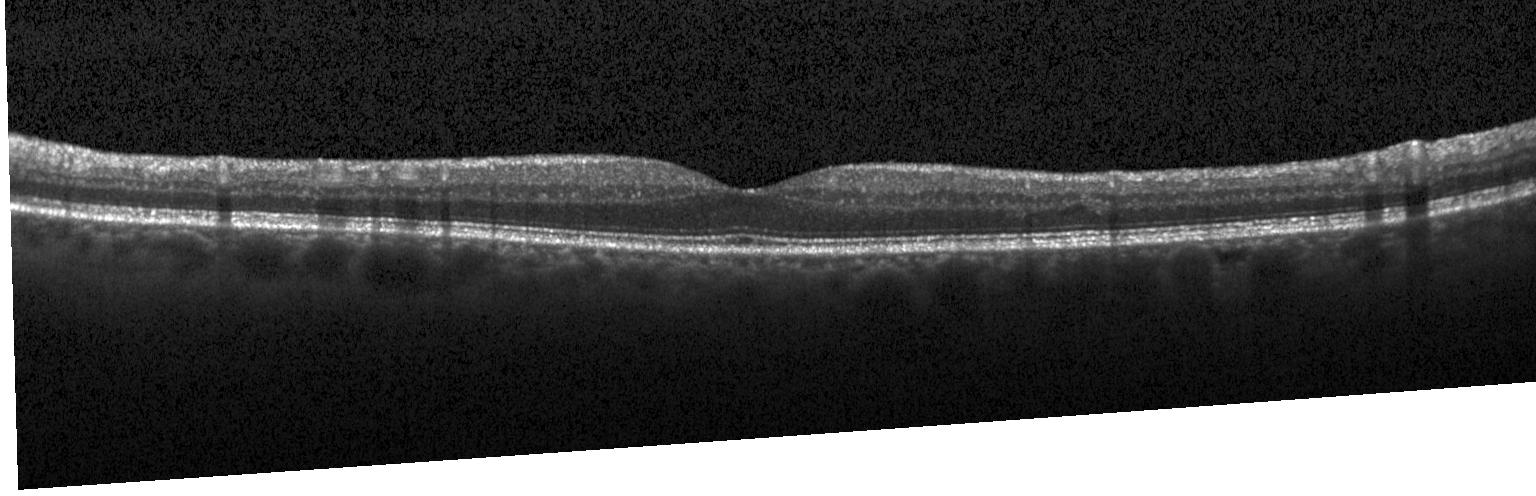

Acquired on a Heidelberg Spectralis; optical coherence tomography B-scan; horizontal scan through the fovea; spectral-domain OCT
Diagnosis: no choroidal neovascularization, no diabetic macular edema, and no drusen.